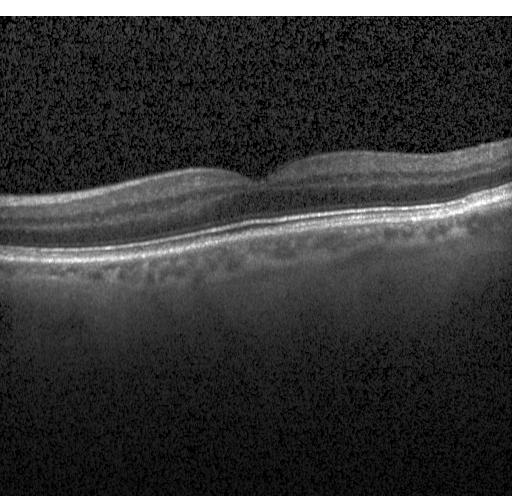
Optical coherence tomography scan. Impression: no evidence of choroidal neovascularization, diabetic macular edema, or drusen.